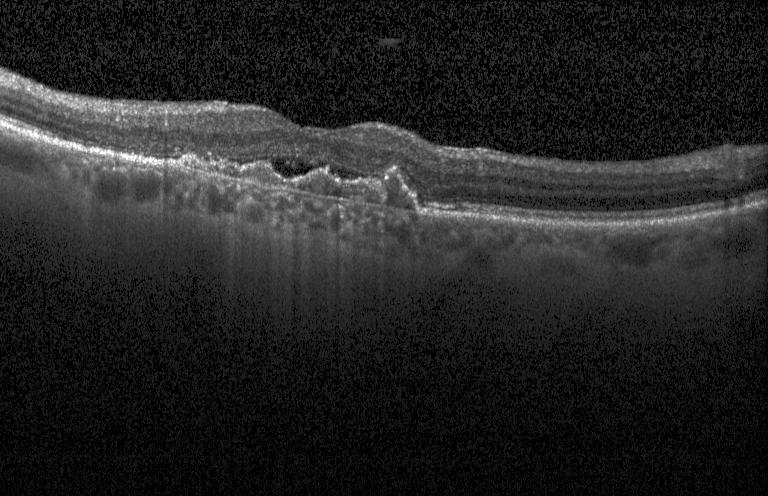
Retinal OCT cross-section showing CNV.